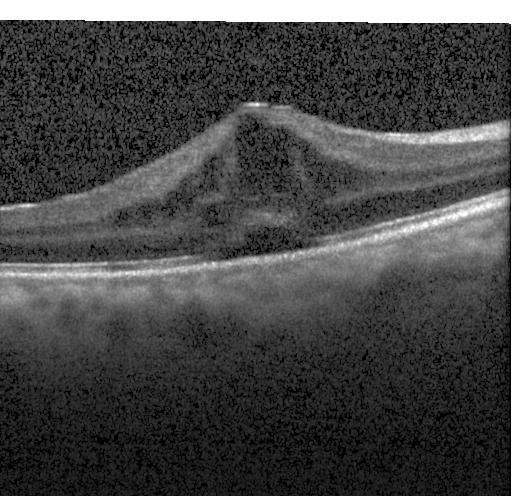 Spectral-domain OCT. Heidelberg Spectralis OCT system. Optical coherence tomography scan.
Impression: DME.